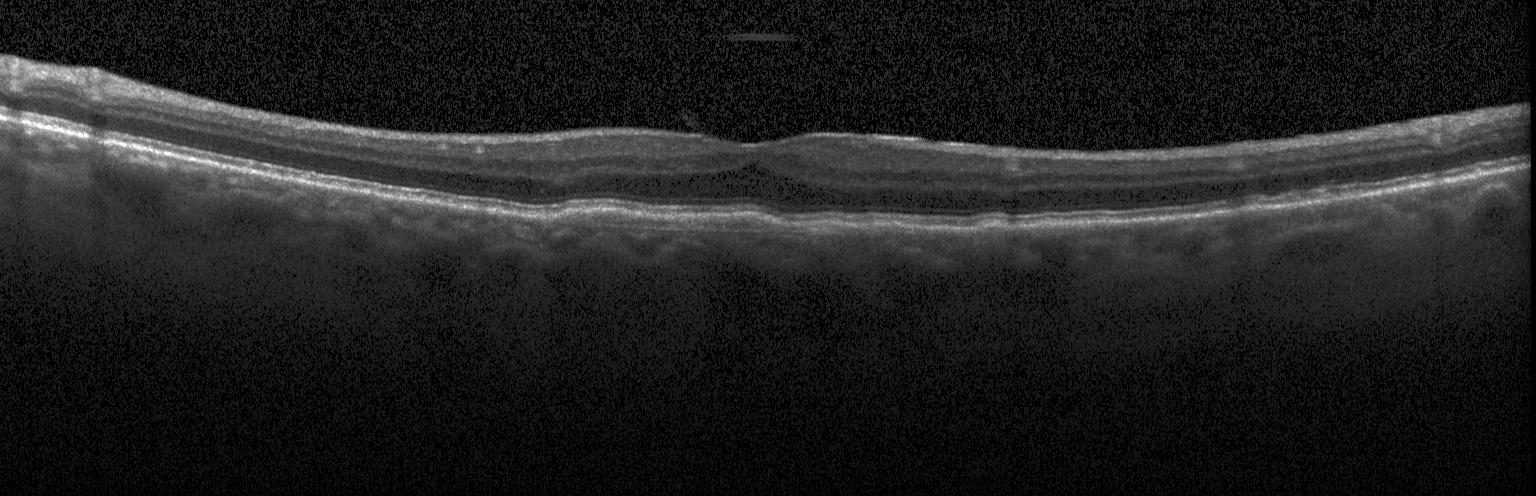 OCT finding: a choroidal neovascular membrane.